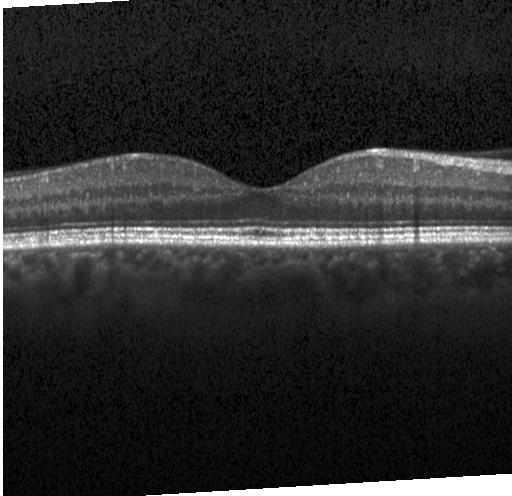

Retinal OCT cross-section showing no choroidal neovascularization, no diabetic macular edema, and no drusen.